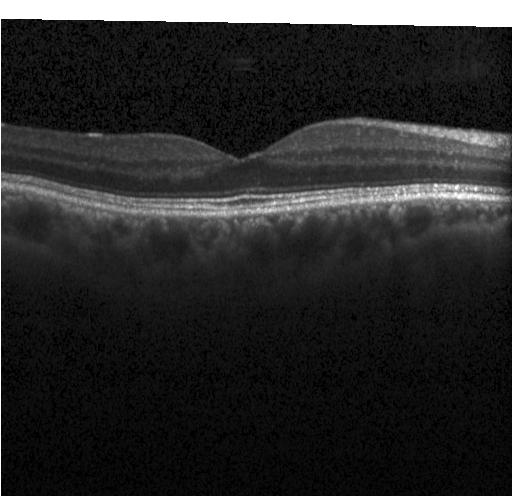
Retinal OCT cross-section; SD-OCT — Finding: no evidence of choroidal neovascularization, diabetic macular edema, or drusen.